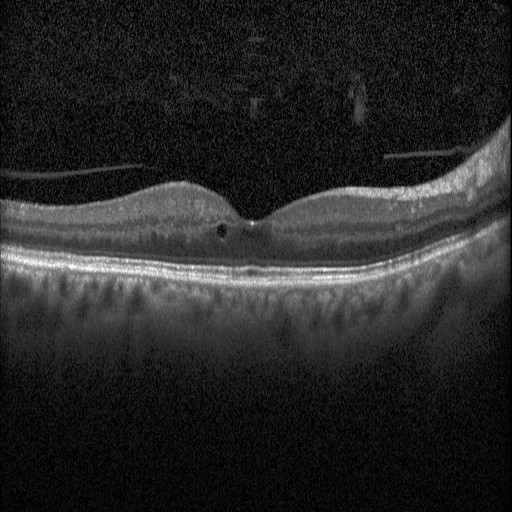
Retinal OCT B-scan. Impression: DME.